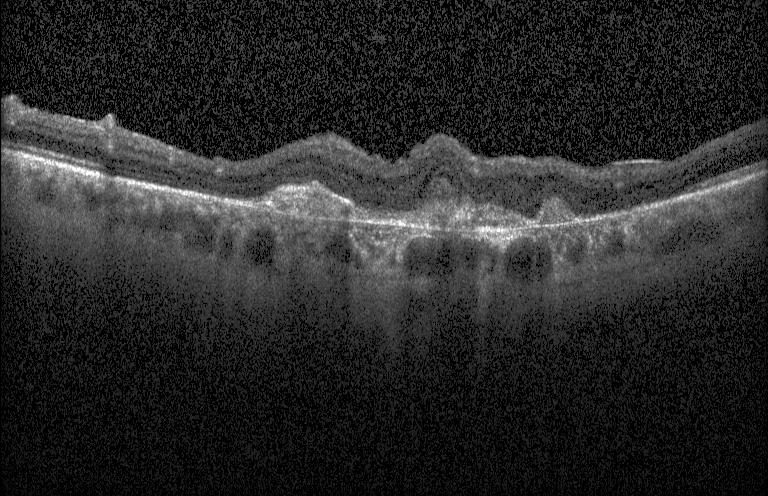
Diagnosis: a choroidal neovascular membrane.